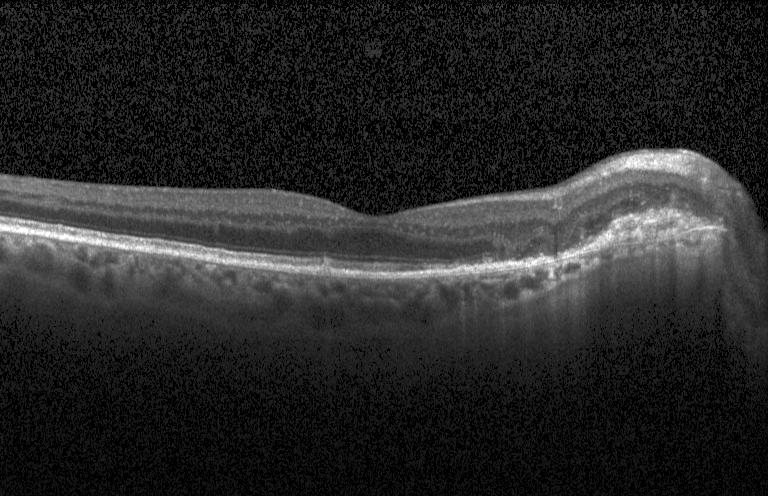

Retinal OCT cross-section
This B-scan demonstrates a choroidal neovascular membrane.